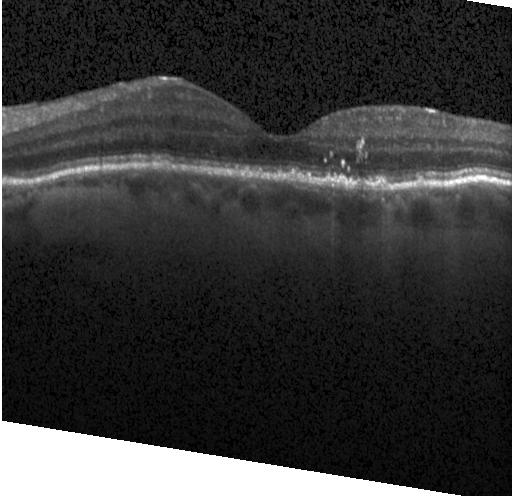

Heidelberg Spectralis OCT system, spectral-domain OCT, OCT line scan.
Drusen.